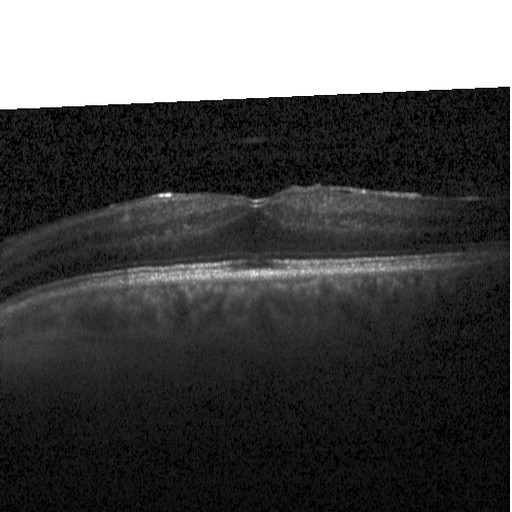 OCT B-scan — OCT finding: diabetic macular edema (DME).